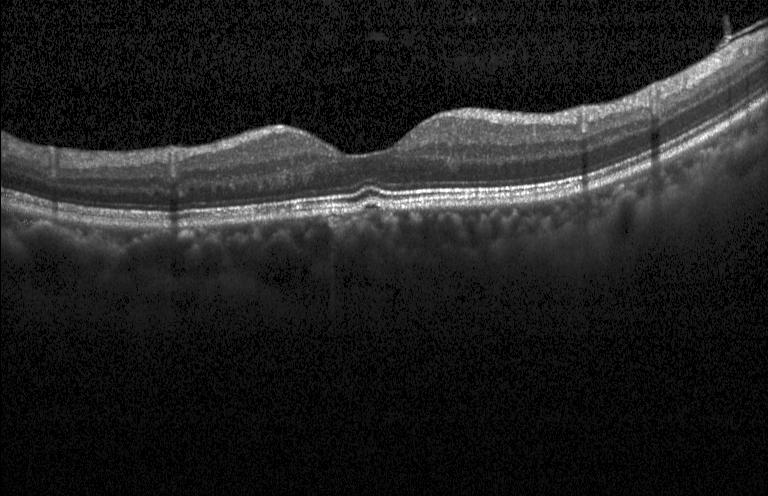
Heidelberg Spectralis. Spectral-domain OCT. OCT line scan. Through the macula
The scan shows no choroidal neovascularization, diabetic macular edema, or drusen.